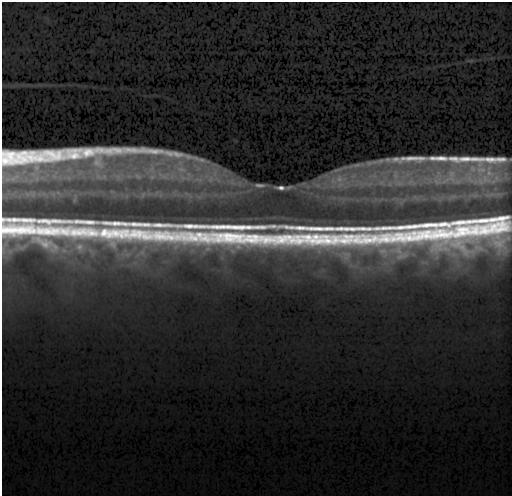

OCT line scan.
Finding: neither choroidal neovascularization, diabetic macular edema, nor drusen.